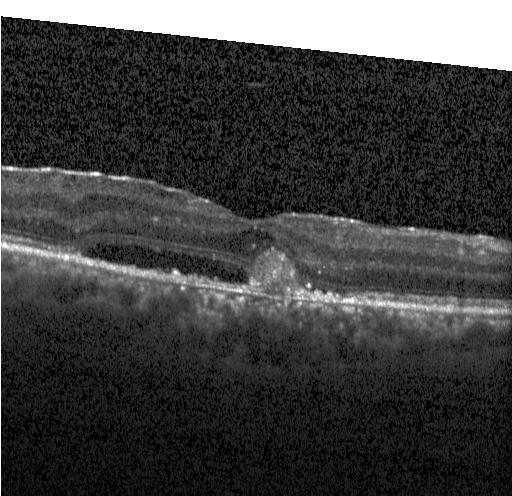
Horizontal scan through the fovea, SD-OCT, retinal OCT cross-section. CNV.